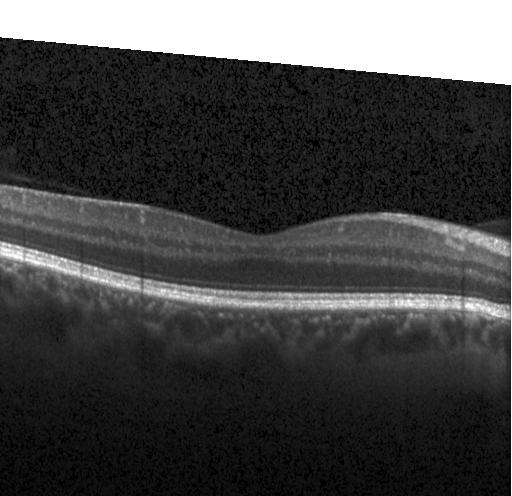

Optical coherence tomography scan
The scan shows no CNV, no DME, and no drusen.